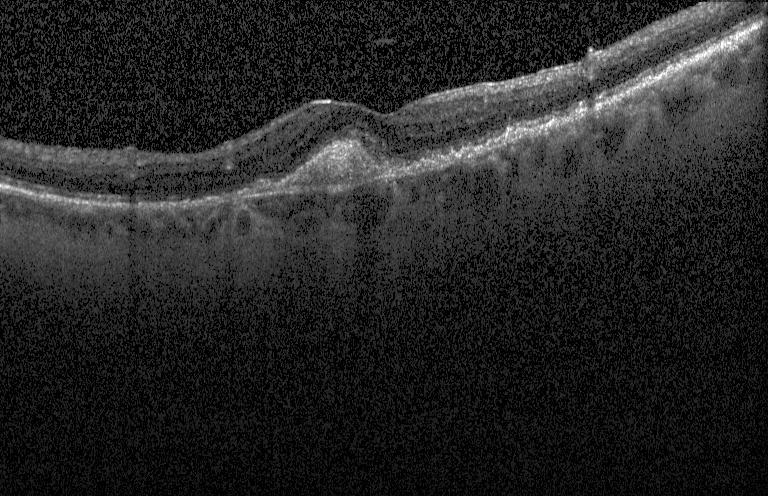
OCT line scan, spectral-domain optical coherence tomography, acquired on a Heidelberg Spectralis.
The scan shows a choroidal neovascular membrane.